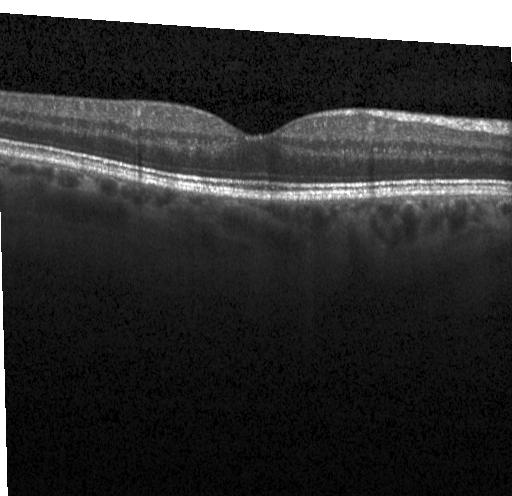
Horizontal scan through the fovea, retinal OCT B-scan. Diagnosis: no choroidal neovascularization, no diabetic macular edema, and no drusen.